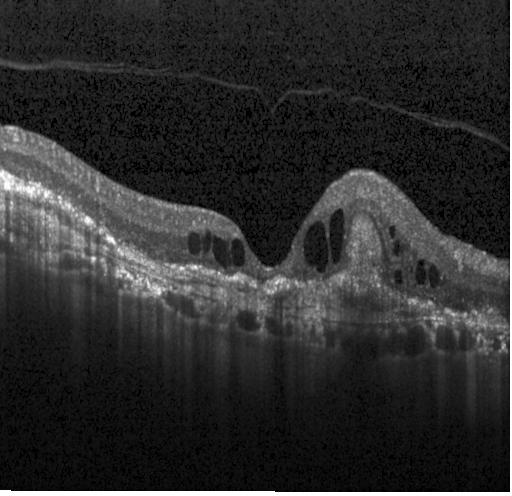
Heidelberg Spectralis OCT system, optical coherence tomography B-scan
OCT finding: a choroidal neovascular membrane.